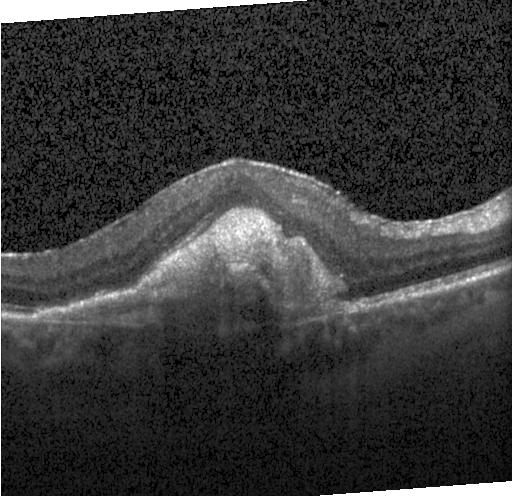 OCT line scan, horizontal scan through the fovea, SD-OCT
Assessment: choroidal neovascularization.